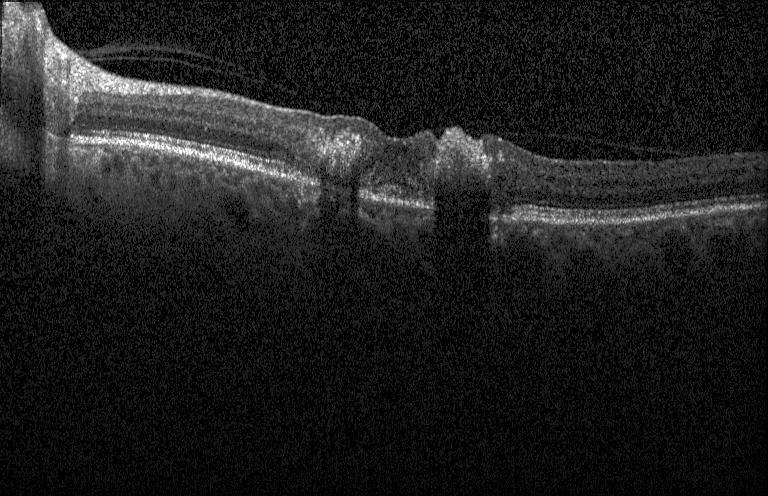

SD-OCT, centered on the fovea, retinal OCT cross-section. Finding: choroidal neovascularization.